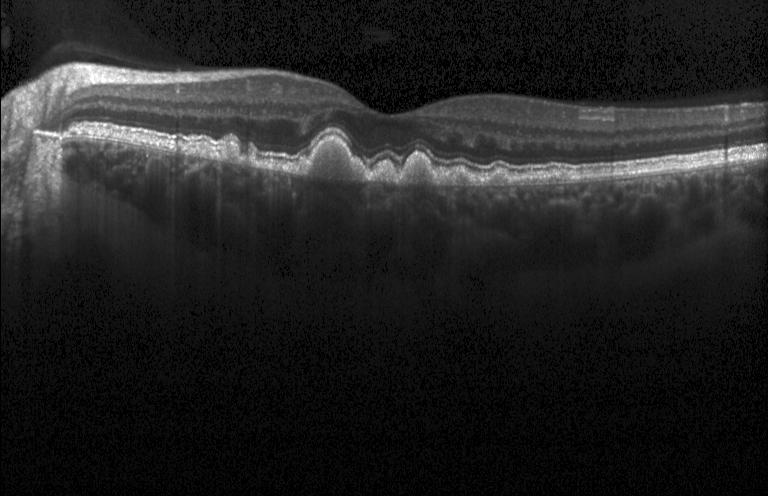
Optical coherence tomography B-scan, spectral-domain optical coherence tomography.
Assessment: multiple drusen.